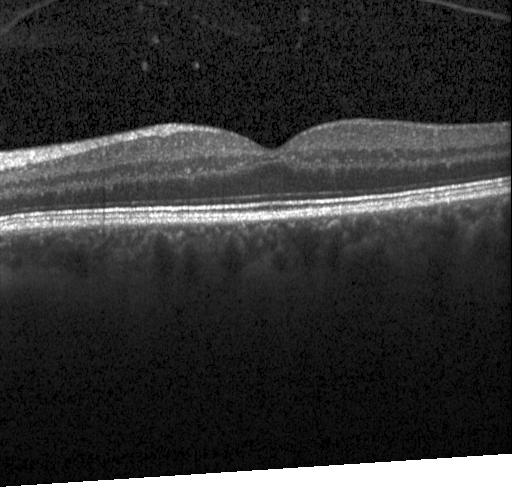

Impression: no evidence of choroidal neovascularization, diabetic macular edema, or drusen.